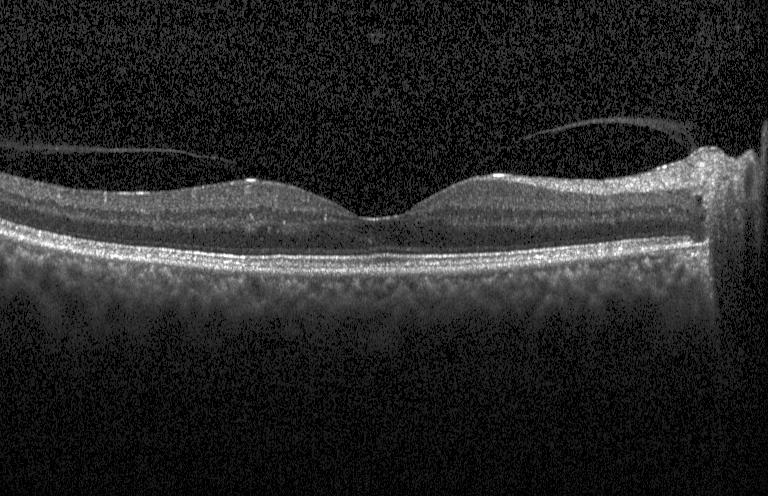

Optical coherence tomography B-scan — Diagnosis: neither choroidal neovascularization, diabetic macular edema, nor drusen.